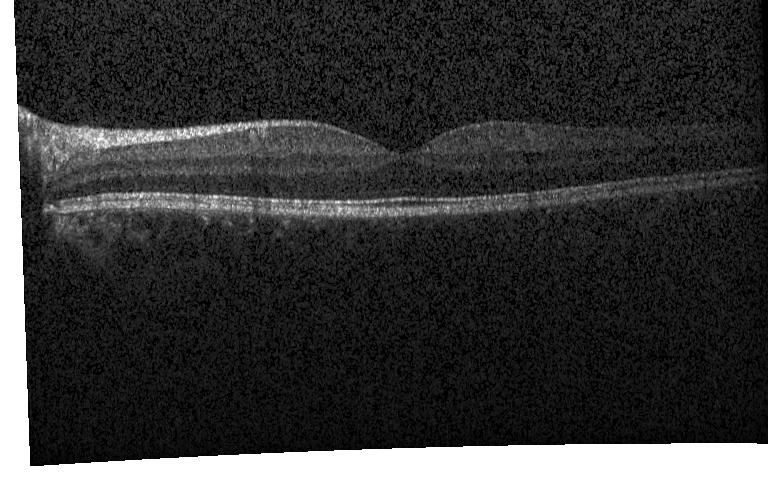
Spectral-domain optical coherence tomography; optical coherence tomography scan; Heidelberg Spectralis OCT system.
Neither CNV, DME, nor drusen.